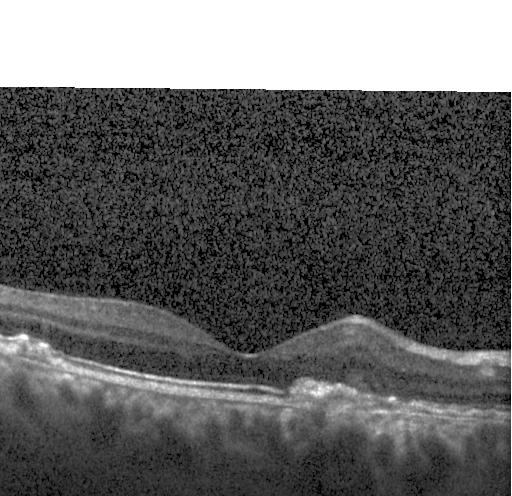

Heidelberg Spectralis OCT system · macular scan · optical coherence tomography scan.
OCT finding: a choroidal neovascular membrane.